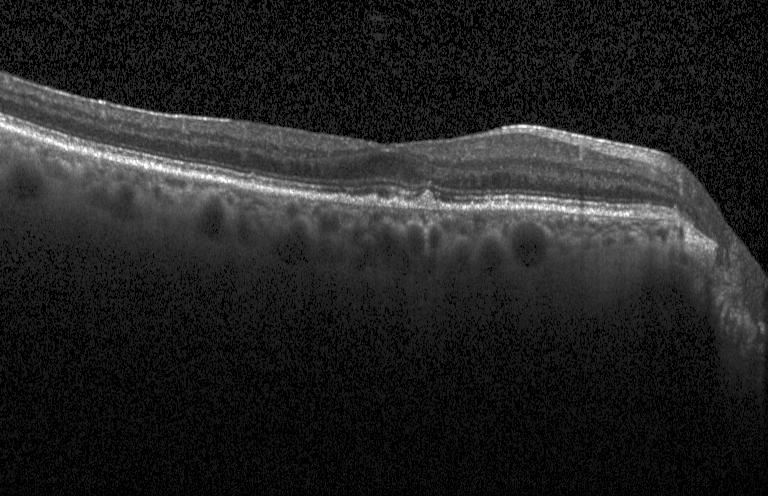
OCT B-scan; spectral-domain OCT.
Diagnosis: sub-RPE drusenoid deposits.